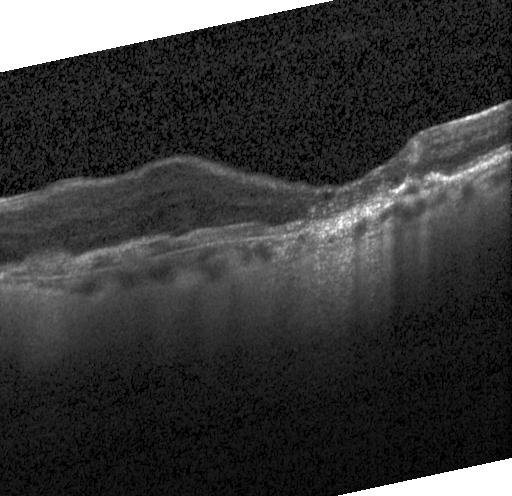
The scan shows a choroidal neovascular membrane.